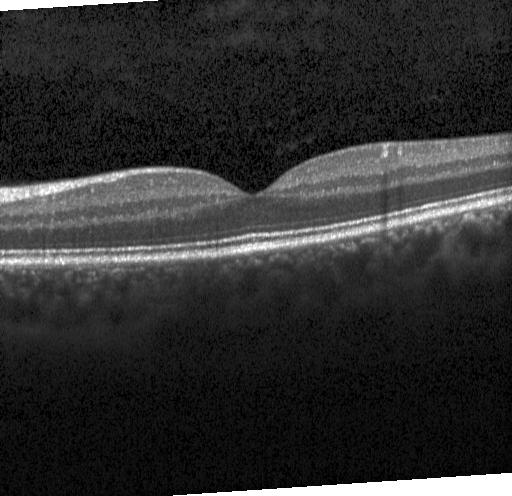 Retinal OCT cross-section showing no choroidal neovascularization, diabetic macular edema, or drusen.